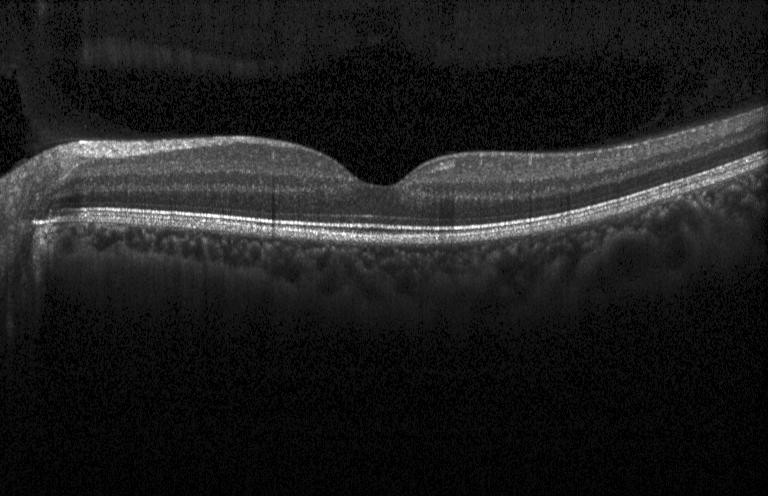 Spectral-domain OCT B-scan: no choroidal neovascularization, diabetic macular edema, or drusen.